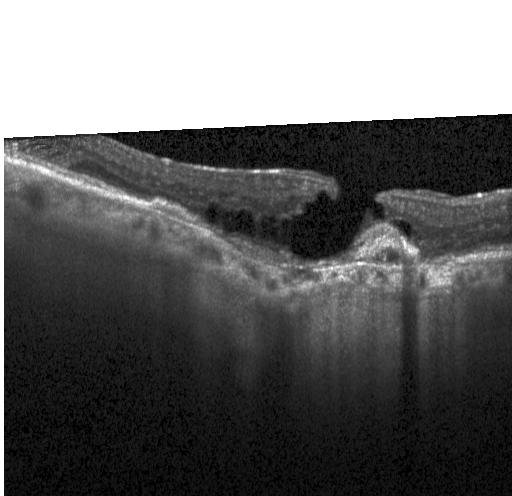
OCT B-scan showing a choroidal neovascular membrane.